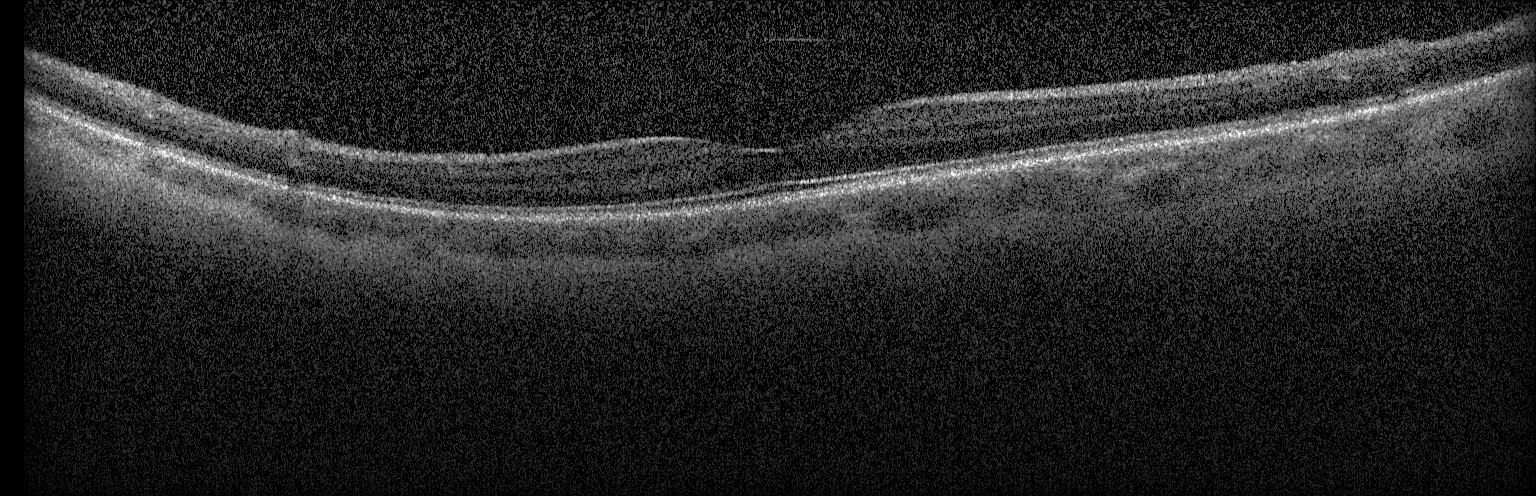 This B-scan demonstrates no evidence of choroidal neovascularization, diabetic macular edema, or drusen.